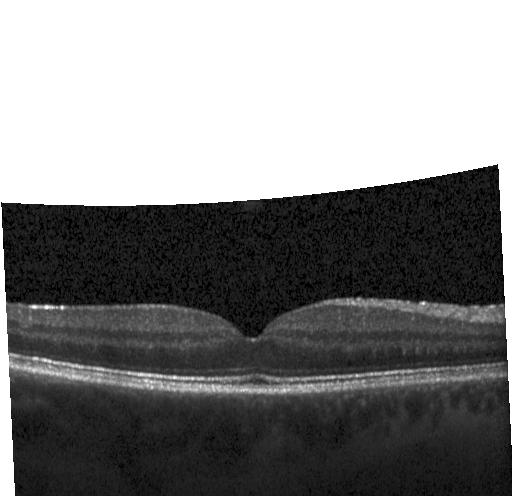
Spectral-domain optical coherence tomography, horizontal scan through the fovea, optical coherence tomography B-scan, acquired on a Heidelberg Spectralis.
Impression: no CNV, no DME, and no drusen.